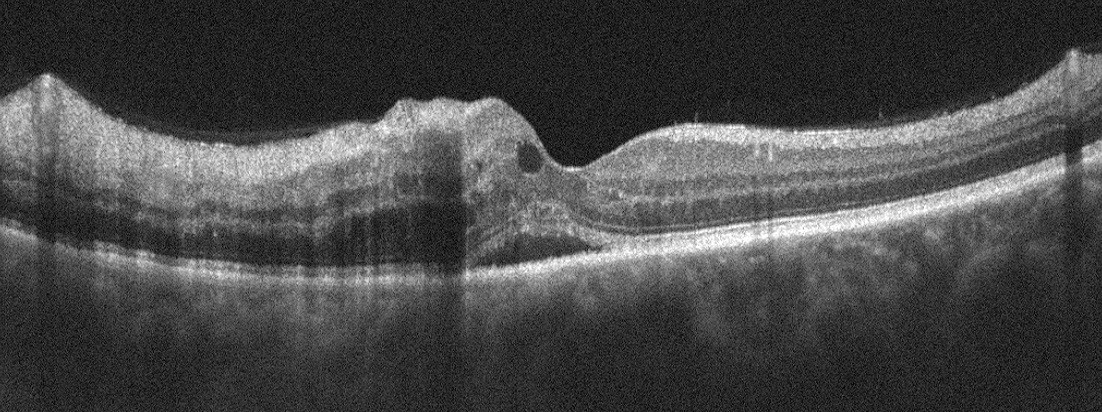
Fovea-centered. Acquired on an Optovue Avanti RTVue XR. Optical coherence tomography scan. RVO.